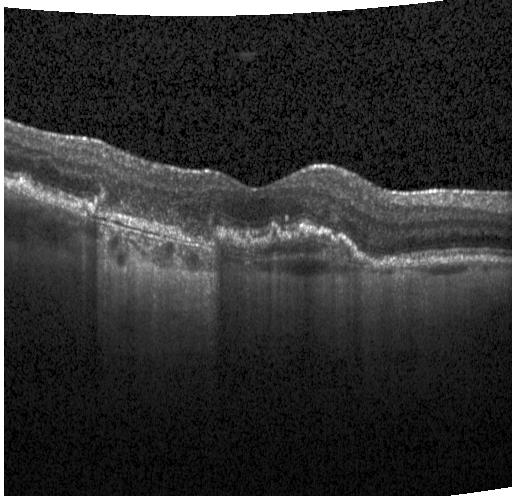

Macular scan. Spectral-domain OCT. Optical coherence tomography B-scan. Choroidal neovascularization (CNV).